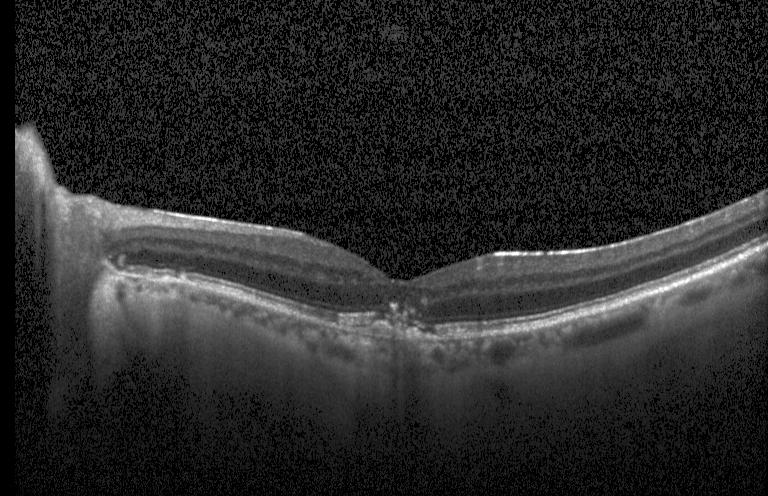 Optical coherence tomography B-scan. Assessment: CNV.